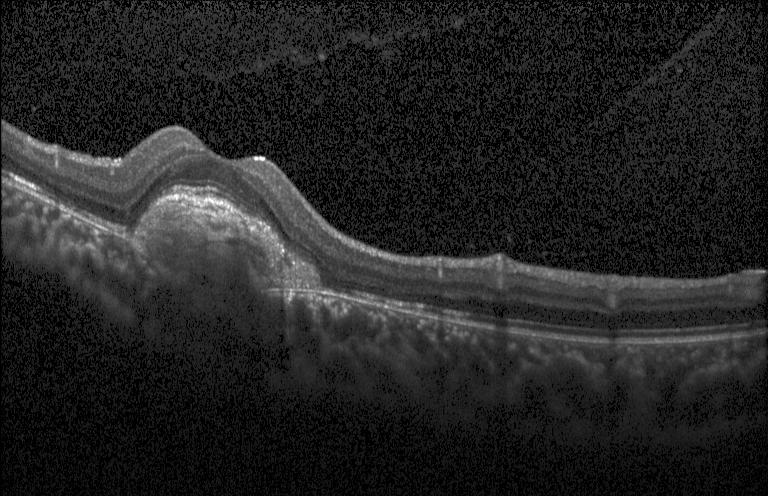 Finding: a choroidal neovascular membrane.